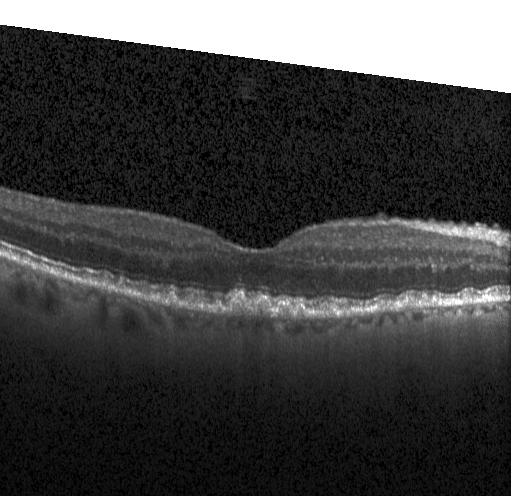
Heidelberg Spectralis, spectral-domain optical coherence tomography, OCT B-scan.
Macular OCT: sub-RPE drusenoid deposits.